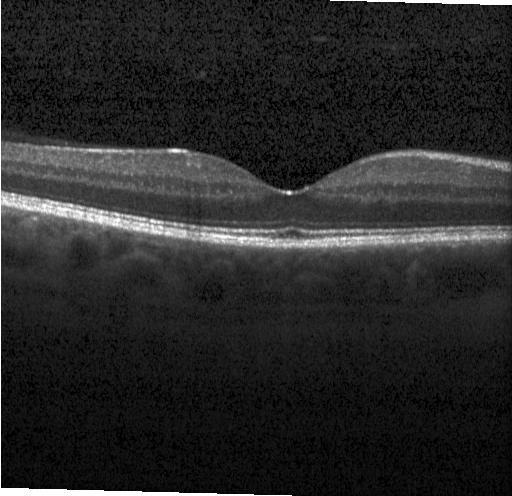

Finding: no CNV, no DME, and no drusen.